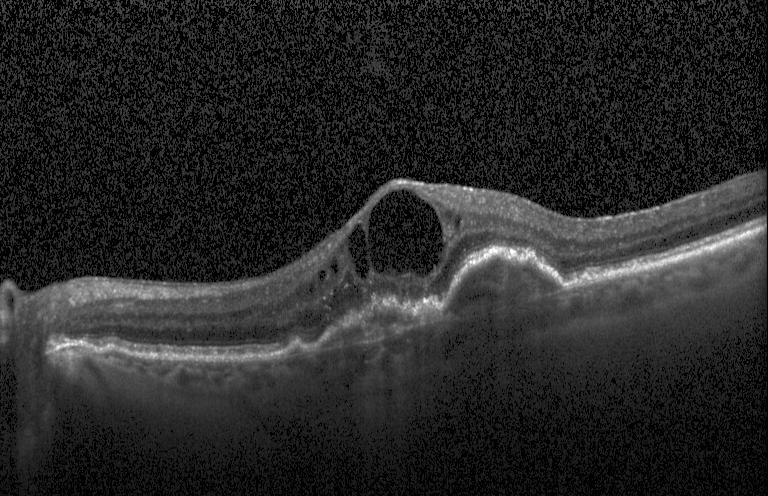 SD-OCT; optical coherence tomography B-scan; macular scan — Impression: CNV.